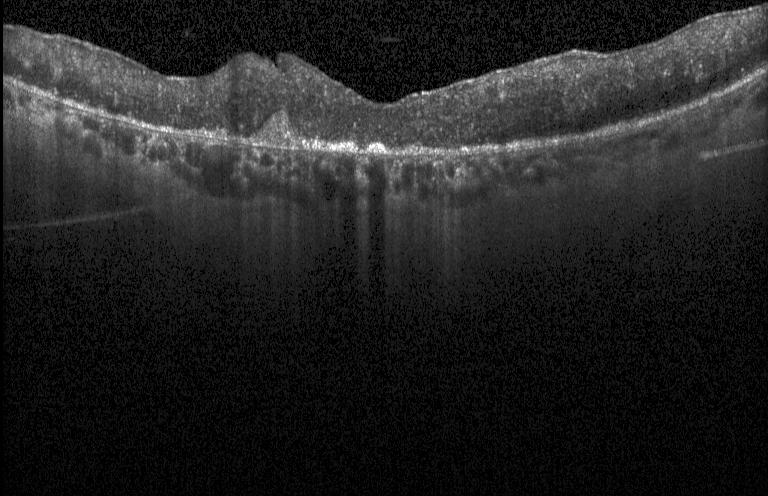
Retinal OCT cross-section; Heidelberg Spectralis OCT system
Finding: a choroidal neovascular membrane.